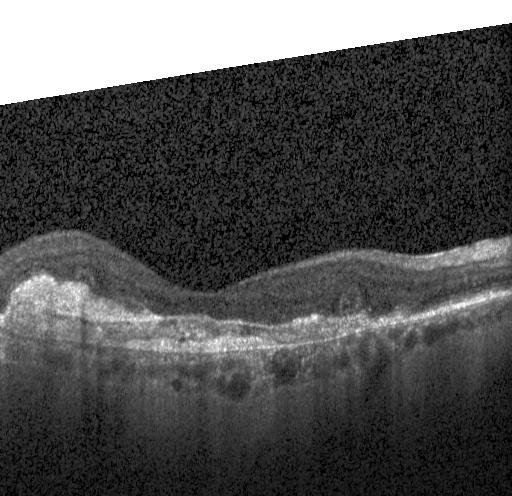

OCT scan showing a choroidal neovascular membrane.